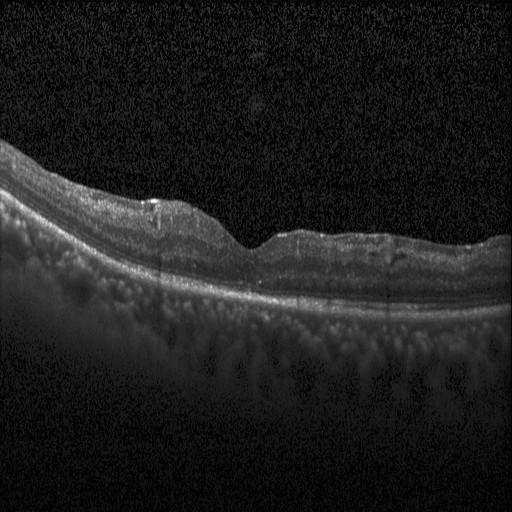 Heidelberg Spectralis OCT system · spectral-domain OCT · macular scan · retinal OCT cross-section — The scan shows diabetic macular edema (DME).